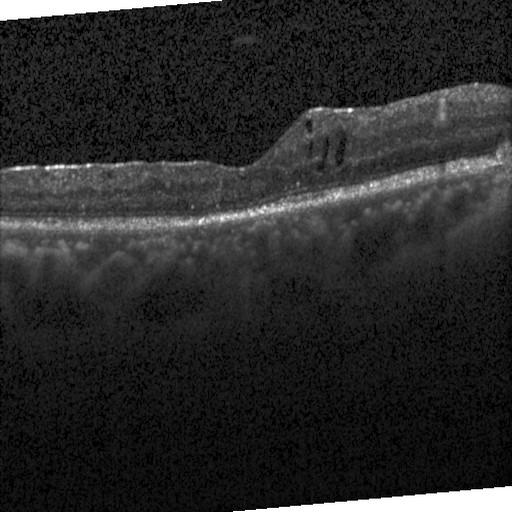 Assessment: DME.